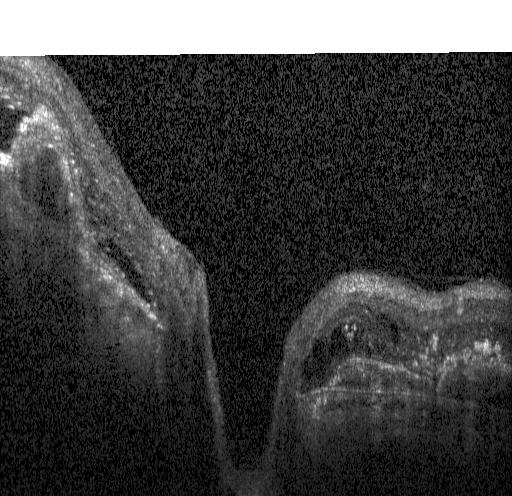 Retinal OCT B-scan
Impression: a choroidal neovascular membrane.